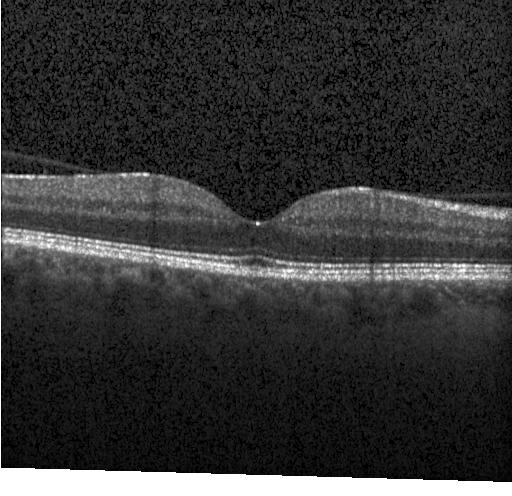
Retinal OCT B-scan. Diagnosis: no choroidal neovascularization, no diabetic macular edema, and no drusen.